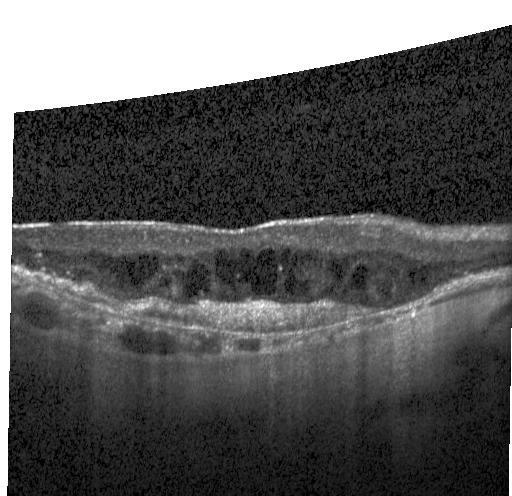
Retinal OCT cross-section · through the macula.
Diagnosis: choroidal neovascularization (CNV).